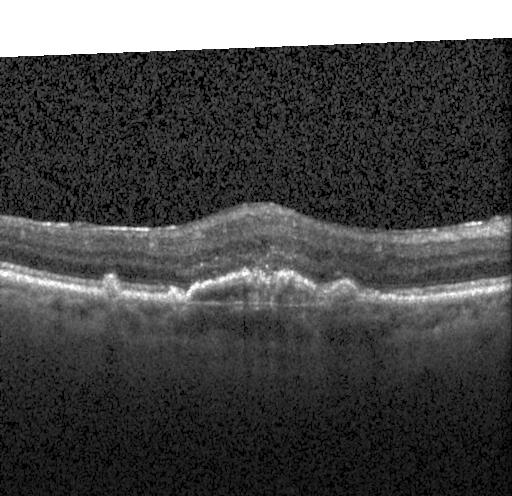 Retinal OCT cross-section showing a choroidal neovascular membrane.